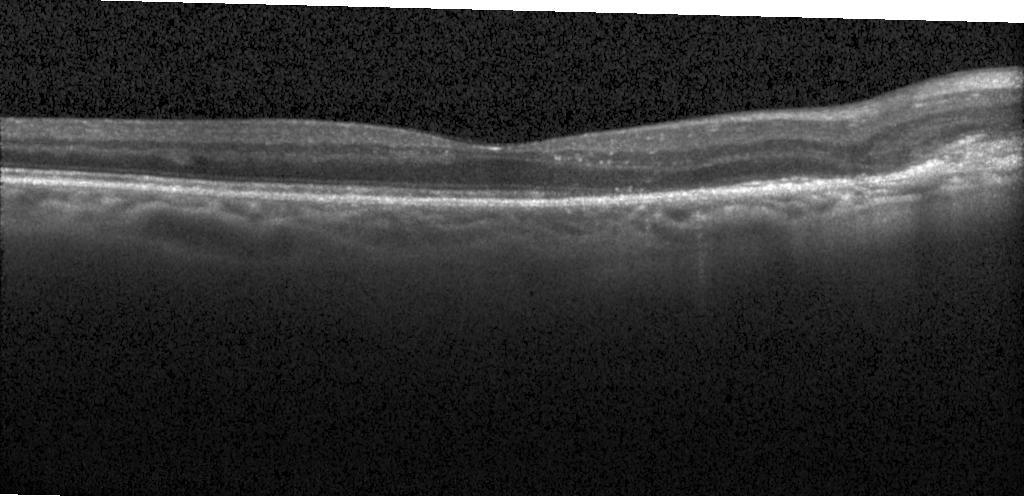
Optical coherence tomography B-scan · spectral-domain optical coherence tomography.
A choroidal neovascular membrane.